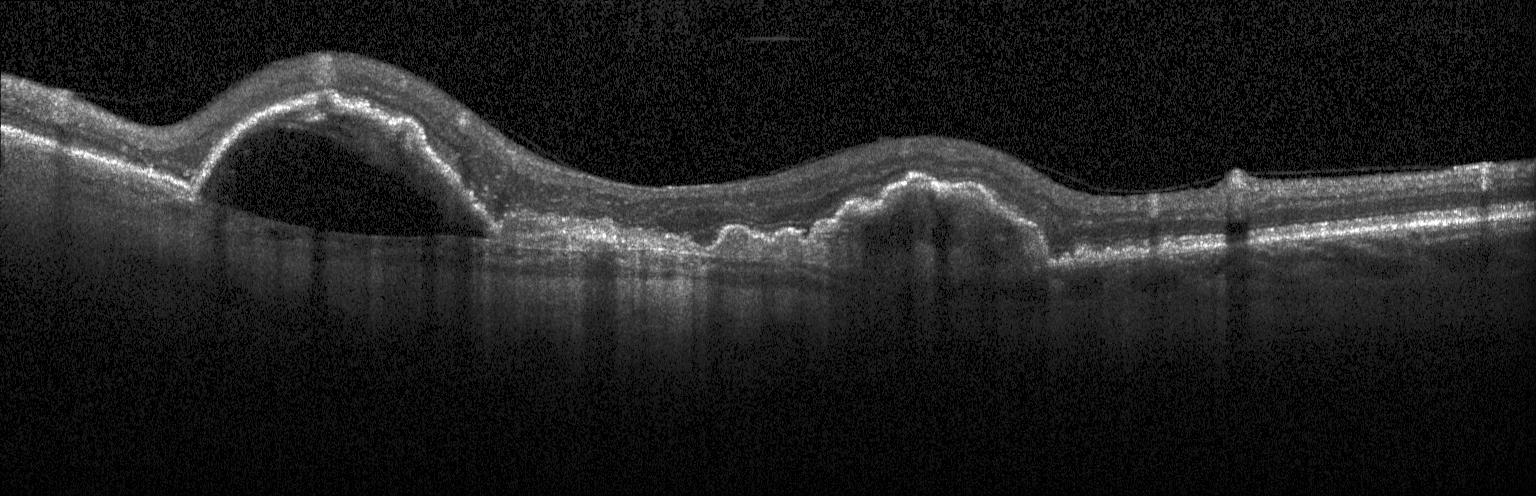 Acquired on a Heidelberg Spectralis. Retinal OCT cross-section. Spectral-domain OCT.
Diagnosis: choroidal neovascularization.